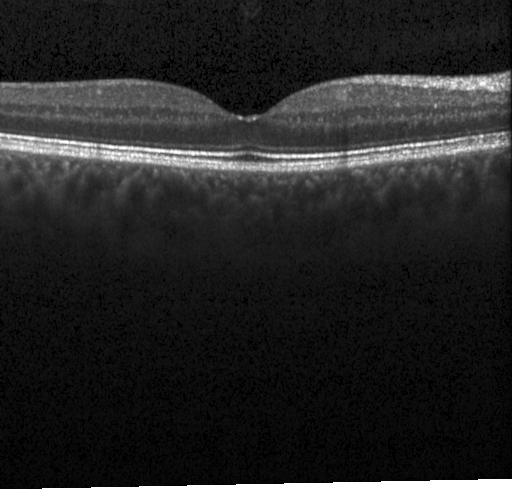 Dx: no CNV, DME, or drusen.